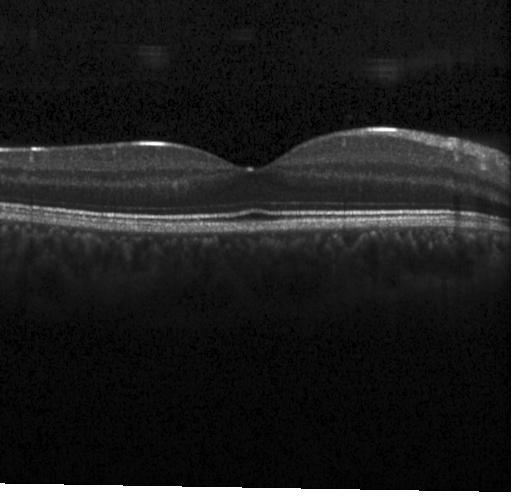
Heidelberg Spectralis OCT system. OCT B-scan — Assessment: neither choroidal neovascularization, diabetic macular edema, nor drusen.